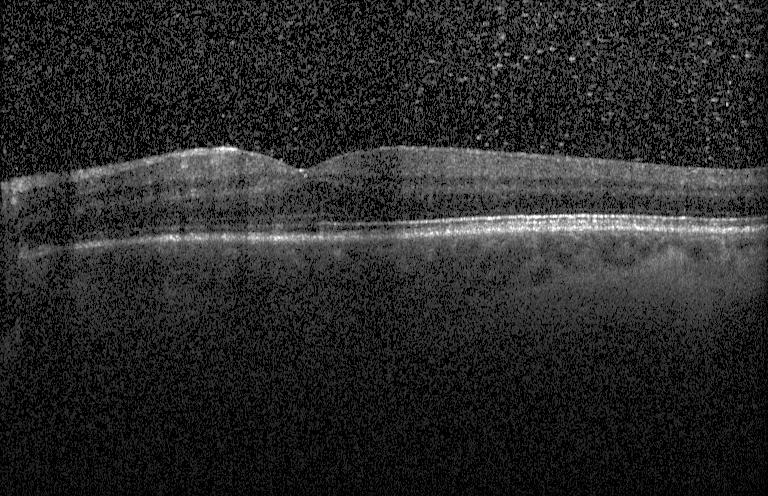

Optical coherence tomography B-scan. Impression: no evidence of choroidal neovascularization, diabetic macular edema, or drusen.